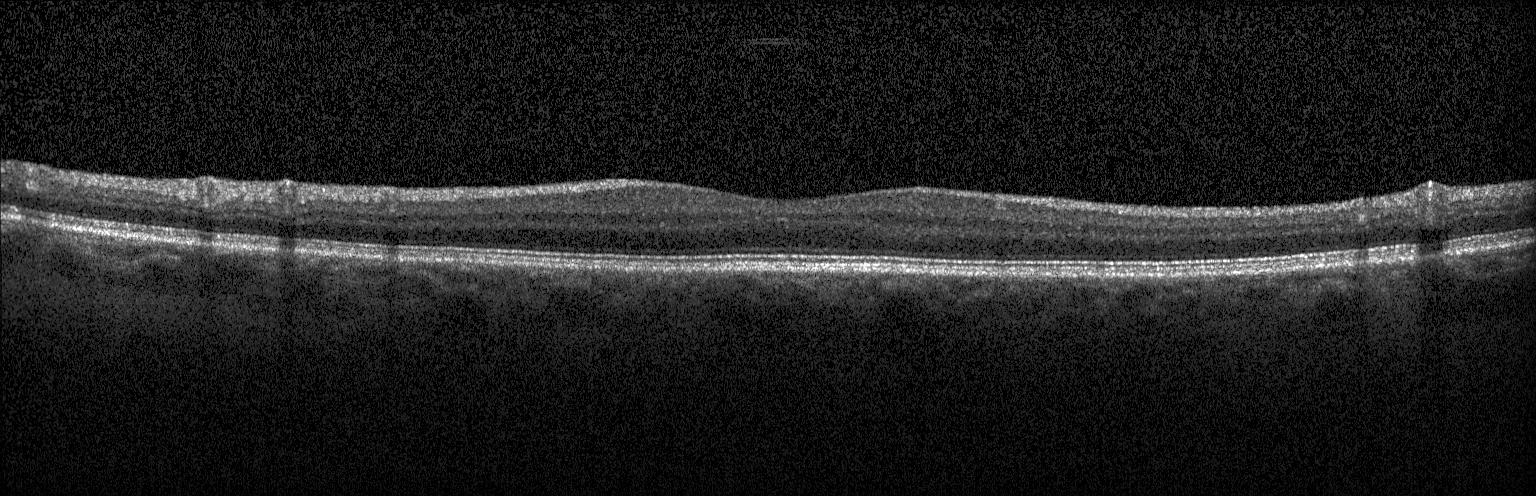

Spectral-domain OCT · retinal OCT B-scan · Heidelberg Spectralis — Finding: no choroidal neovascularization, no diabetic macular edema, and no drusen.